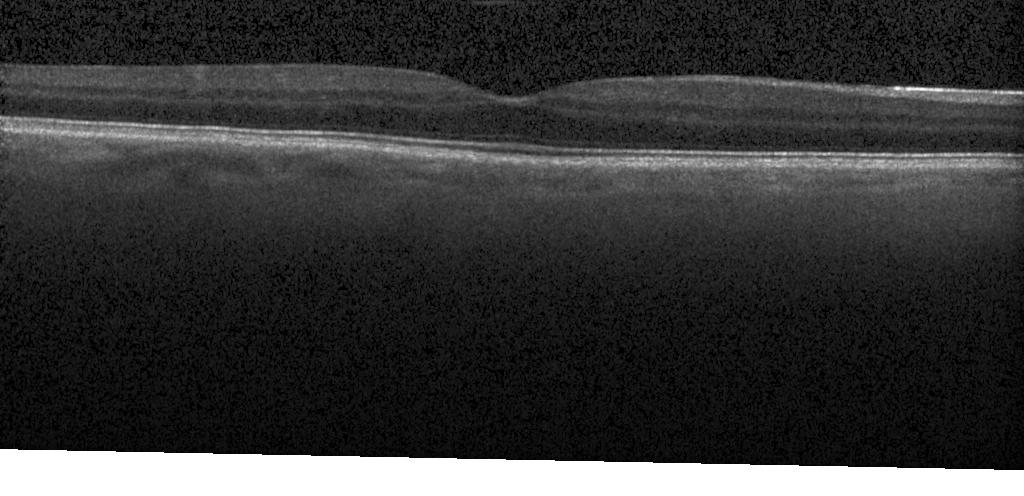

Retinal OCT cross-section — OCT finding: neither CNV, DME, nor drusen.